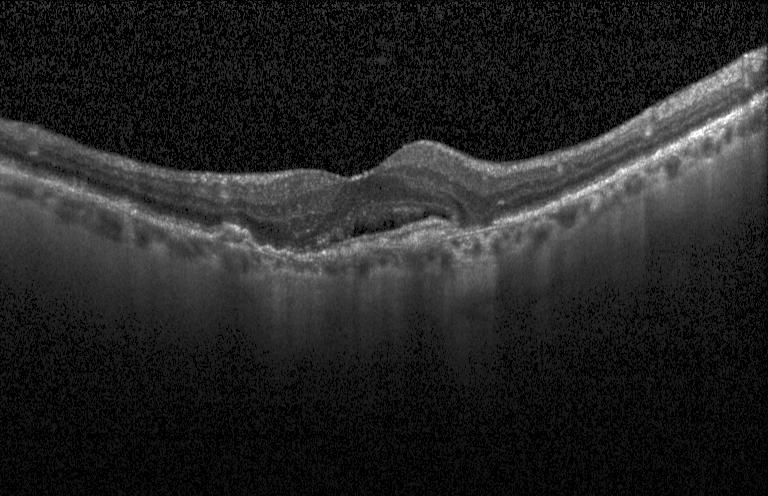

Diagnosis: choroidal neovascularization.